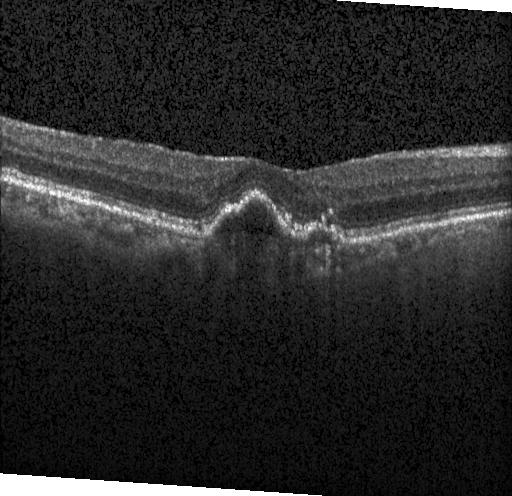
Spectral-domain optical coherence tomography. OCT B-scan. Centered on the fovea
Finding: CNV.